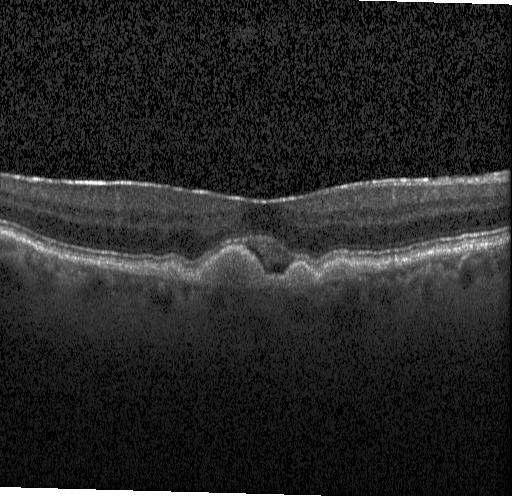 Instrument: Heidelberg Spectralis, retinal OCT B-scan.
The scan shows sub-RPE drusenoid deposits.